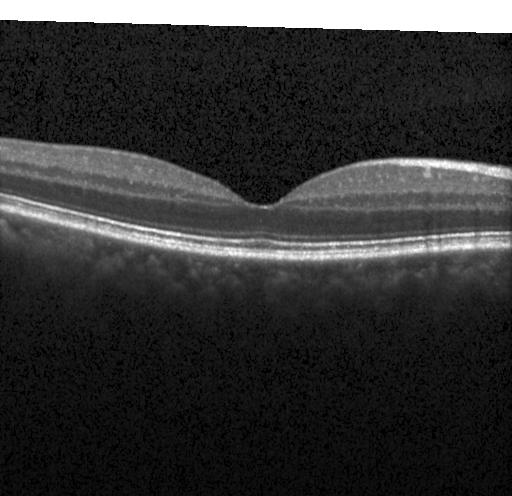
OCT B-scan. Instrument: Heidelberg Spectralis. Spectral-domain optical coherence tomography. Through the macula — Impression: neither choroidal neovascularization, diabetic macular edema, nor drusen.